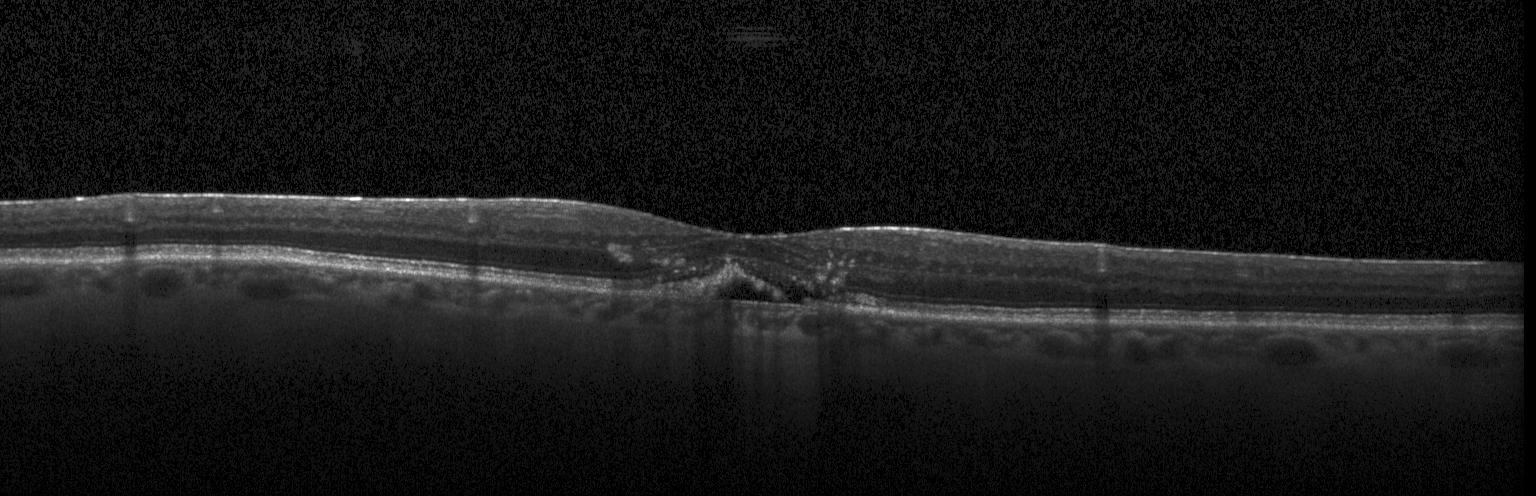 Optical coherence tomography B-scan; Heidelberg Spectralis OCT system; through the macula.
A choroidal neovascular membrane.